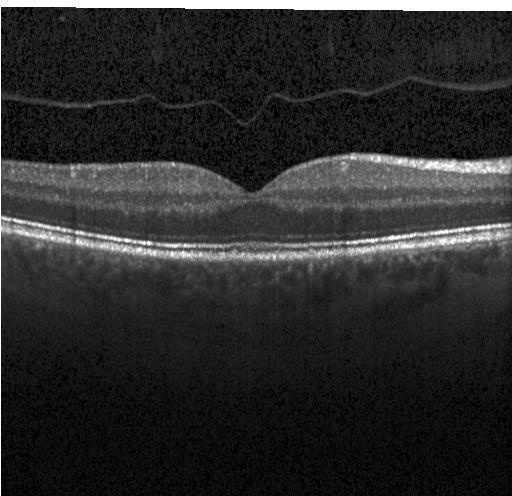
Retinal OCT B-scan
Assessment: no evidence of choroidal neovascularization, diabetic macular edema, or drusen.